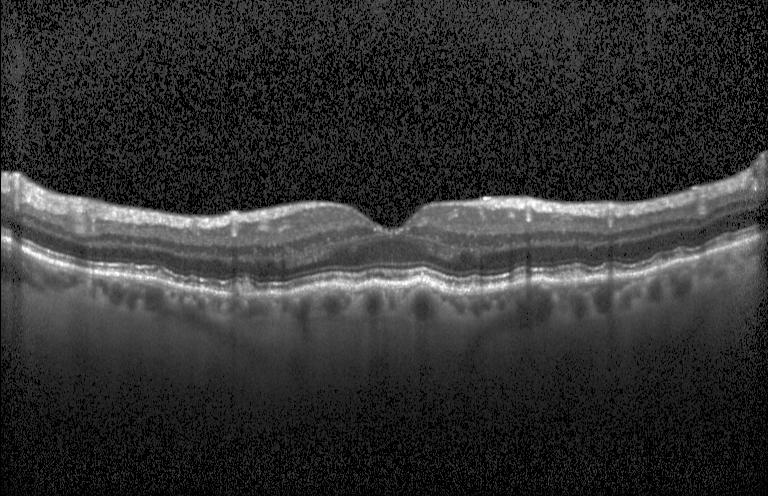 Diagnosis: drusen.